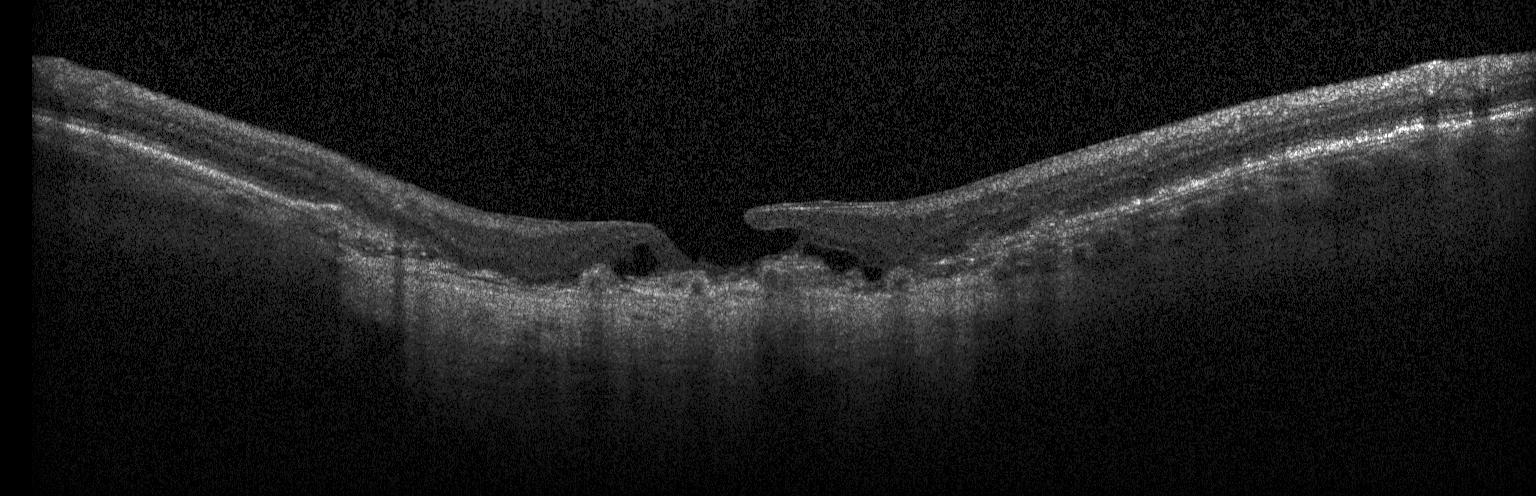
Fovea-centered · spectral-domain optical coherence tomography · Heidelberg Spectralis OCT system · retinal OCT B-scan. A choroidal neovascular membrane.